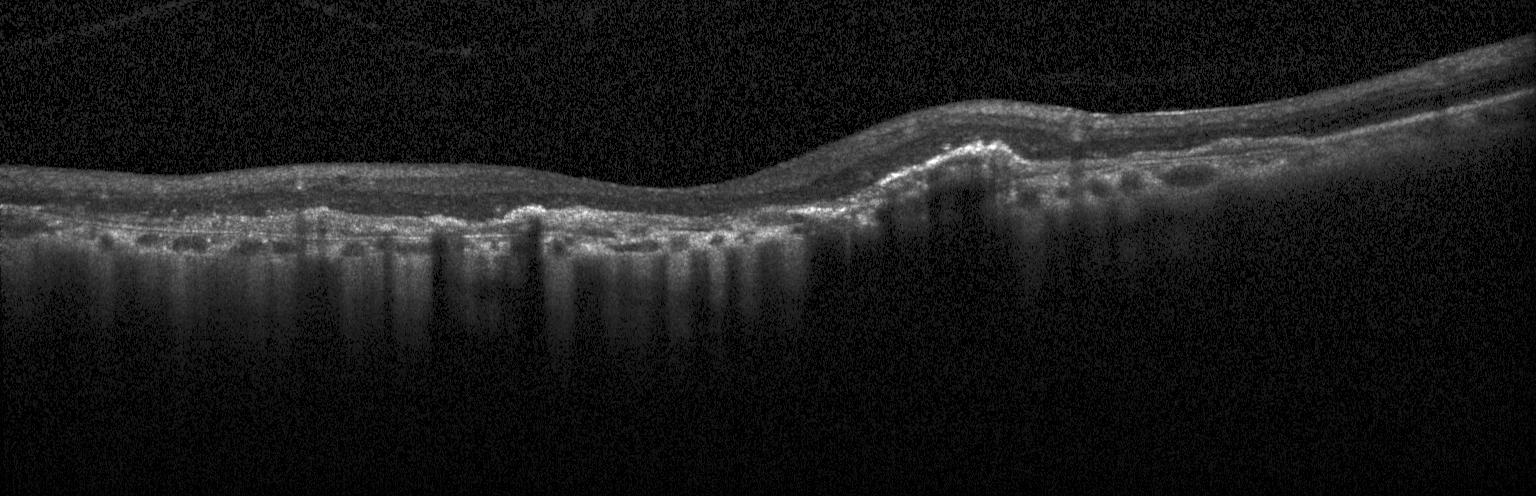

Spectral-domain OCT; OCT B-scan; Heidelberg Spectralis OCT system.
Impression: choroidal neovascularization (CNV).